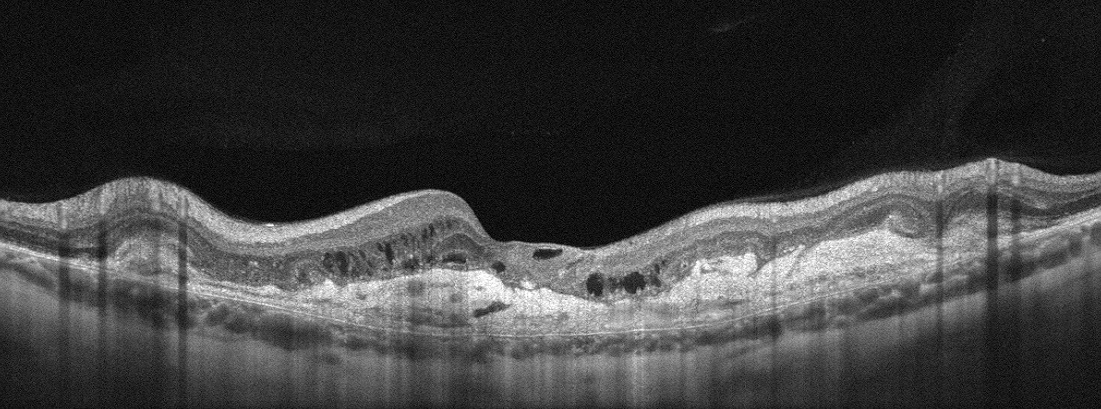 OCT line scan; Optovue Avanti RTVue XR — Diagnosis: age-related macular degeneration (AMD).